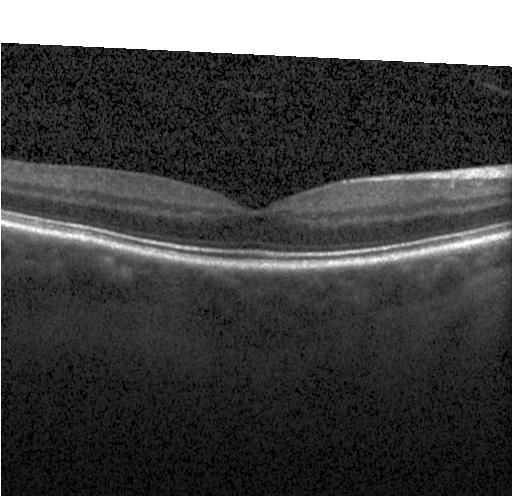 OCT line scan
Diagnosis: no evidence of choroidal neovascularization, diabetic macular edema, or drusen.